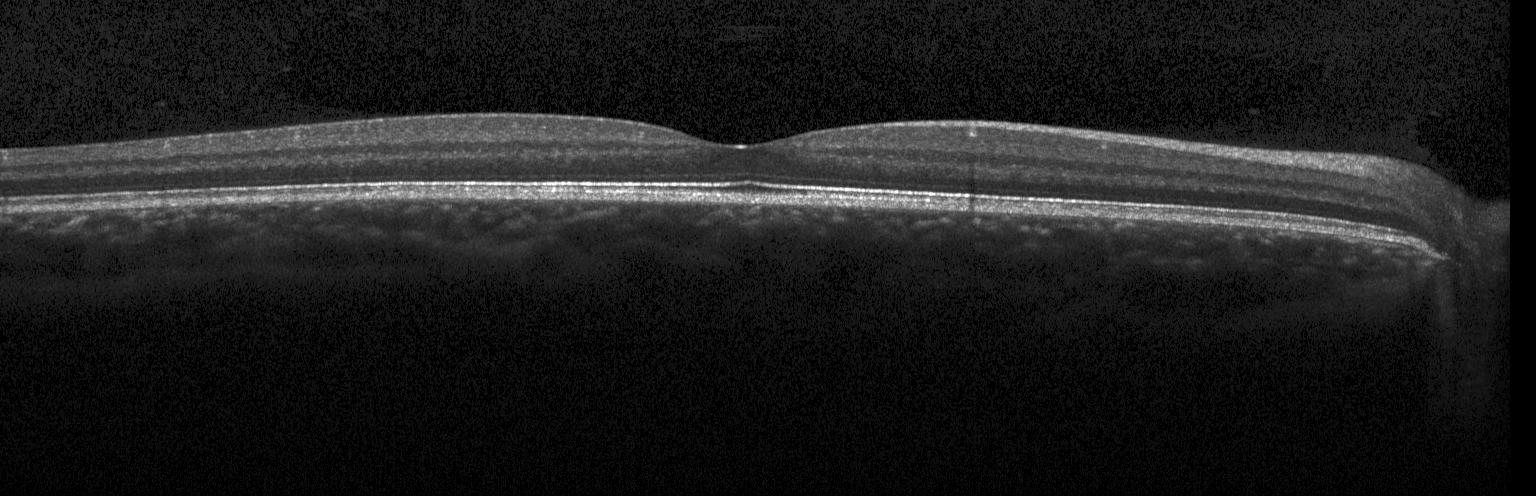

Acquired on a Heidelberg Spectralis, retinal OCT cross-section, centered on the fovea, spectral-domain optical coherence tomography.
The scan shows neither choroidal neovascularization, diabetic macular edema, nor drusen.